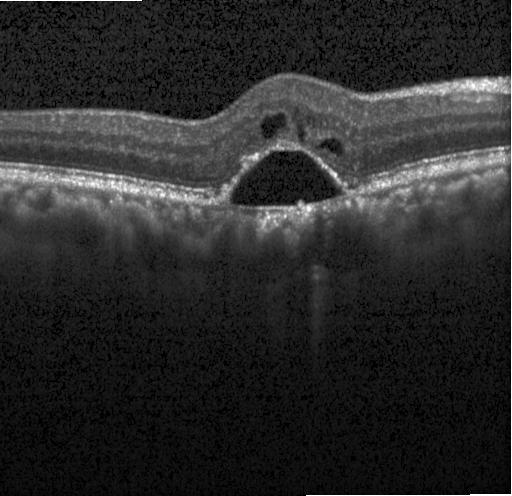 This B-scan demonstrates a choroidal neovascular membrane.